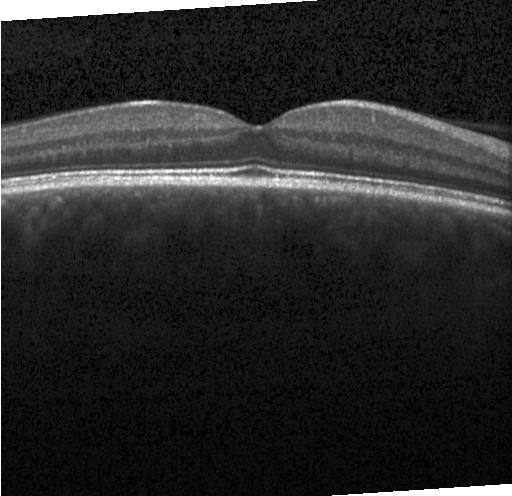

Through the macula. Optical coherence tomography scan. Spectral-domain optical coherence tomography
This B-scan demonstrates no choroidal neovascularization, no diabetic macular edema, and no drusen.